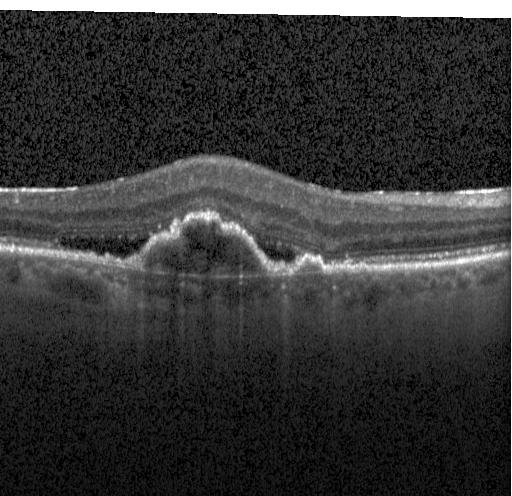 OCT B-scan · macular scan. Diagnosis: choroidal neovascularization.